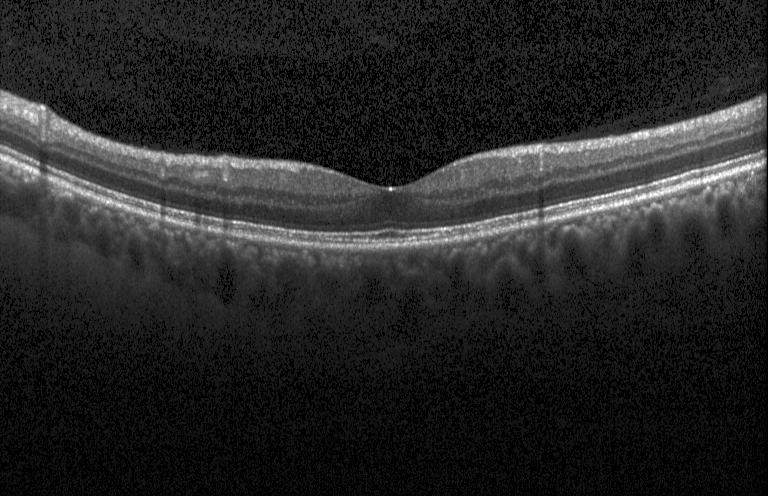

Optical coherence tomography B-scan; Heidelberg Spectralis; spectral-domain optical coherence tomography — Dx: no choroidal neovascularization, no diabetic macular edema, and no drusen.